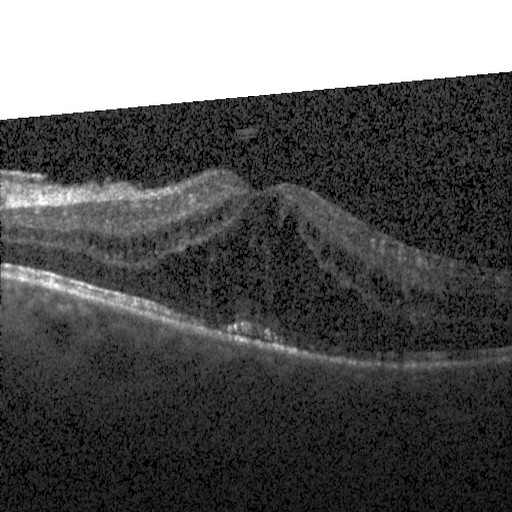
Finding: diabetic macular edema (DME).